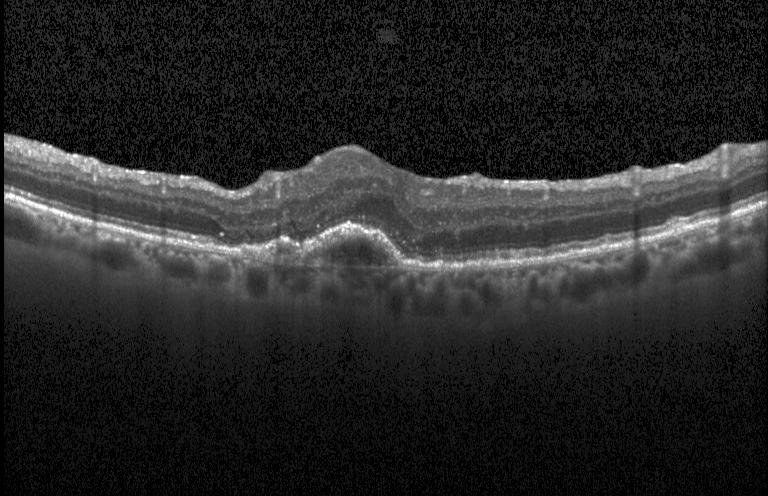

Optical coherence tomography B-scan · acquired on a Heidelberg Spectralis · spectral-domain OCT. This B-scan demonstrates a choroidal neovascular membrane.